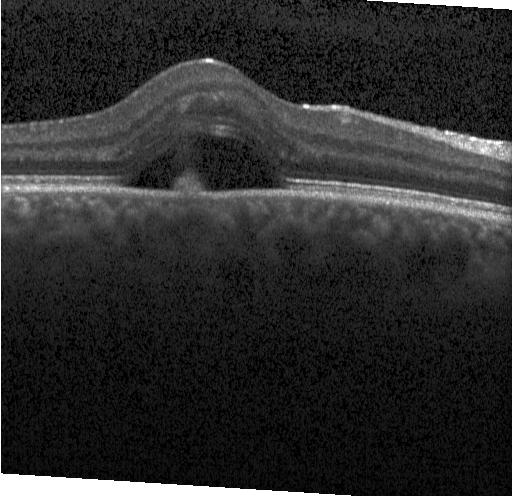
Retinal OCT cross-section. Diagnosis: a choroidal neovascular membrane.